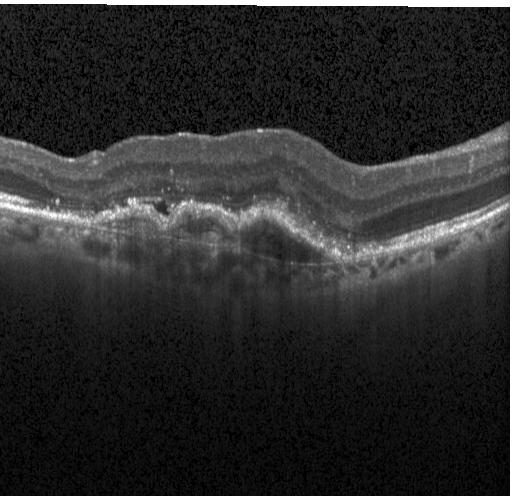
Acquired on a Heidelberg Spectralis · optical coherence tomography B-scan.
The scan shows CNV.